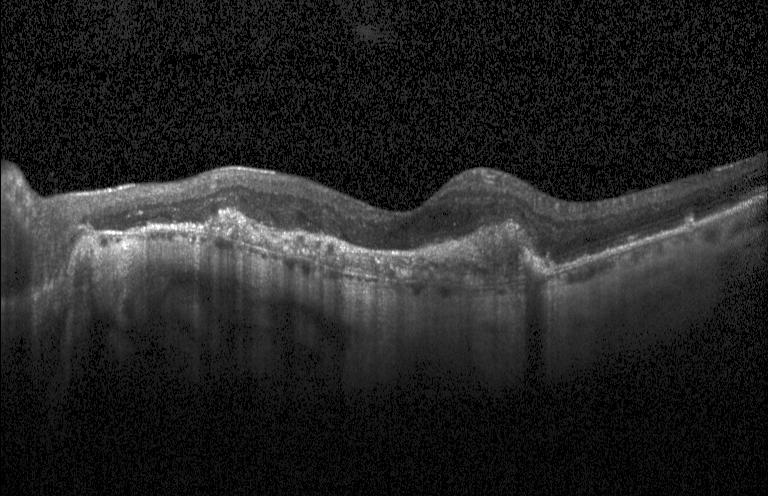

Dx: CNV.